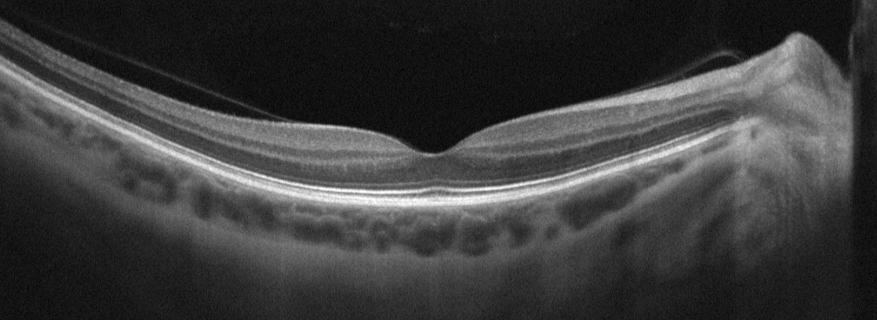

Retinal OCT cross-section.
Assessment: absence of AMD, DME, ERM, RAO, RVO, and vitreomacular interface disease.